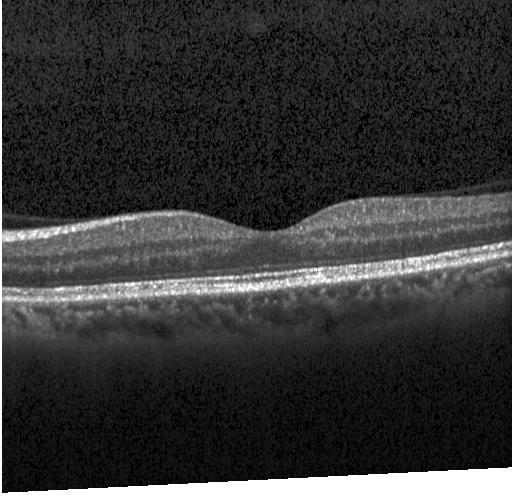
Retinal OCT B-scan; Heidelberg Spectralis; spectral-domain OCT; fovea-centered — This B-scan demonstrates no CNV, no DME, and no drusen.